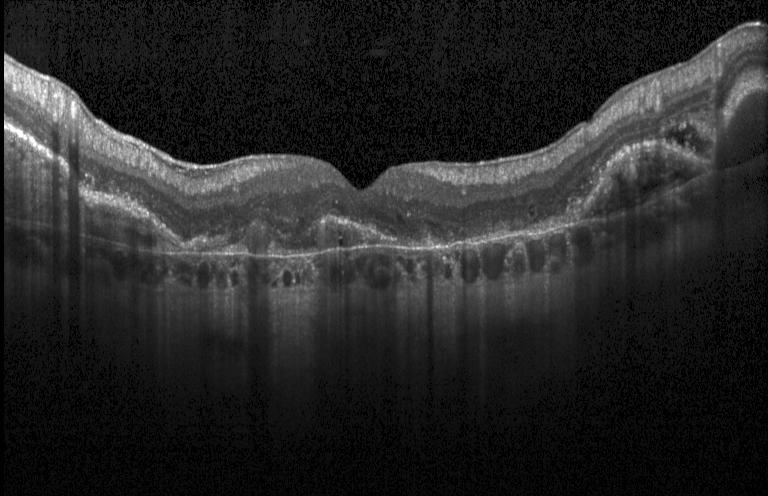
Spectral-domain optical coherence tomography; horizontal scan through the fovea; optical coherence tomography scan — Finding: choroidal neovascularization.